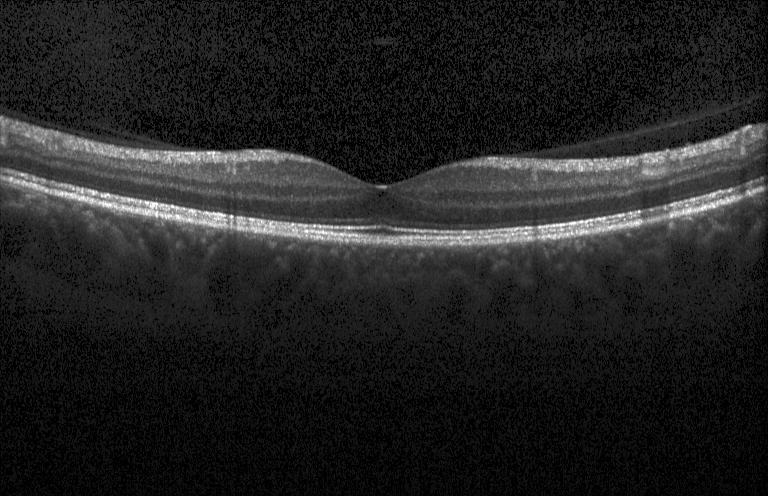
OCT finding: no choroidal neovascularization, diabetic macular edema, or drusen.